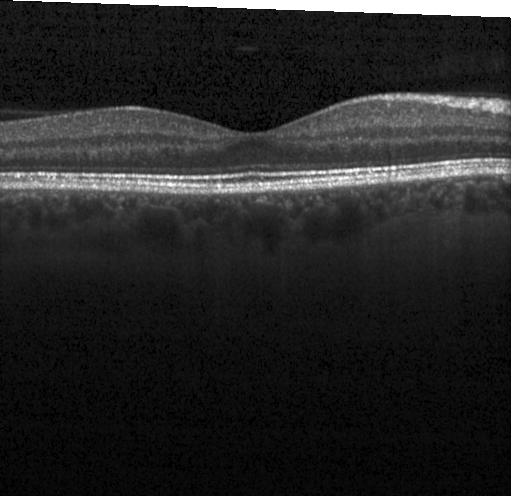 Fovea-centered. Heidelberg Spectralis. Optical coherence tomography B-scan — Finding: neither choroidal neovascularization, diabetic macular edema, nor drusen.